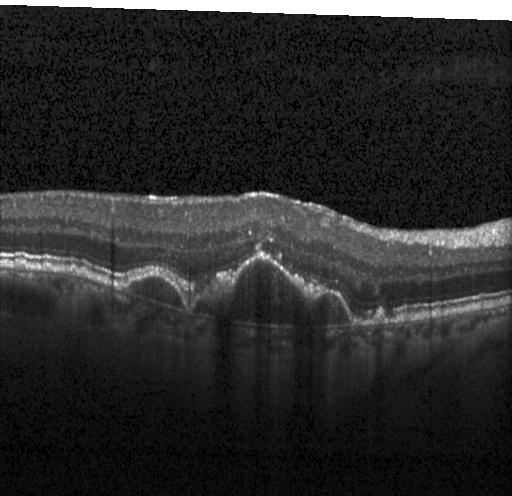

Macular OCT demonstrating CNV.